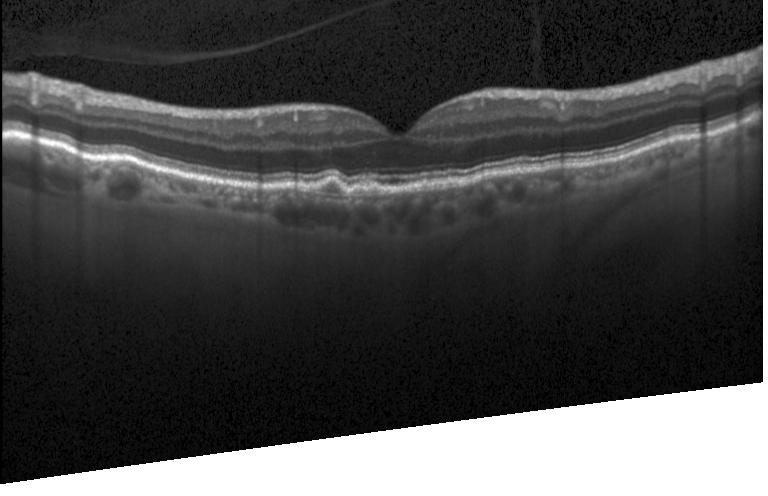 Macular scan. Retinal OCT B-scan. Heidelberg Spectralis. Spectral-domain optical coherence tomography. This B-scan demonstrates multiple drusen.